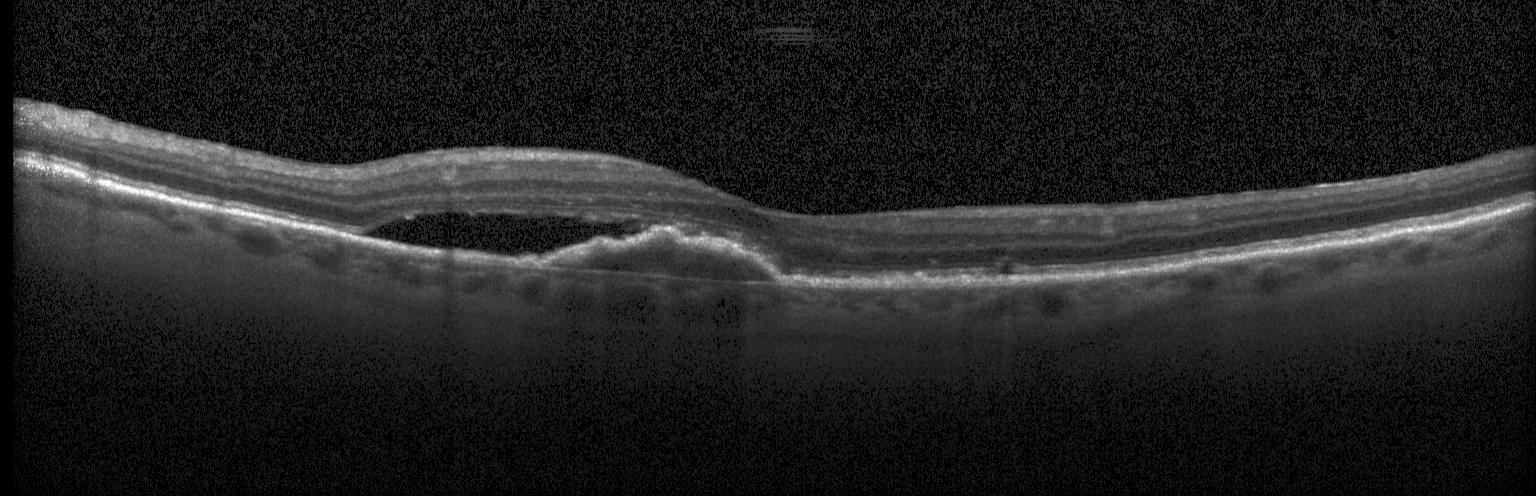
Finding: a choroidal neovascular membrane.